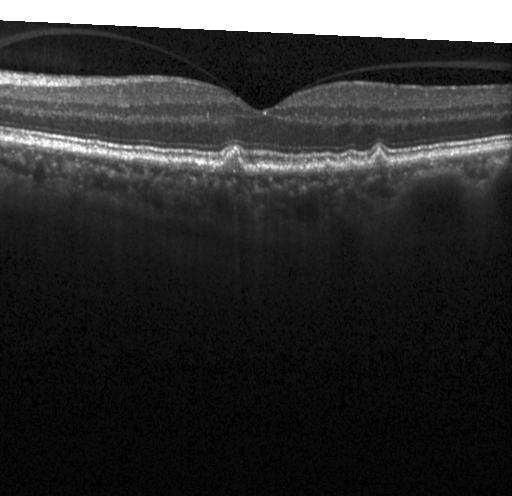
Acquired on a Heidelberg Spectralis · retinal OCT cross-section
Finding: multiple drusen.